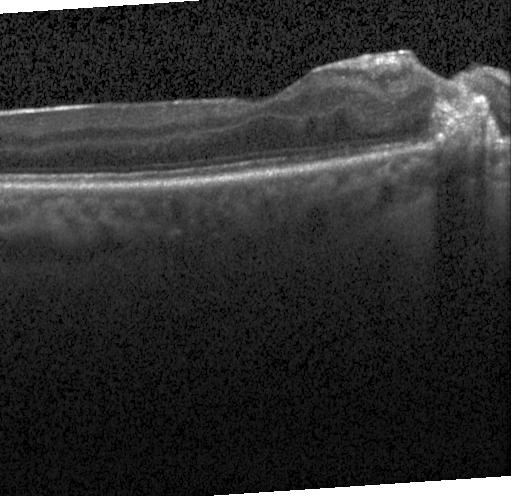
Finding: choroidal neovascularization.